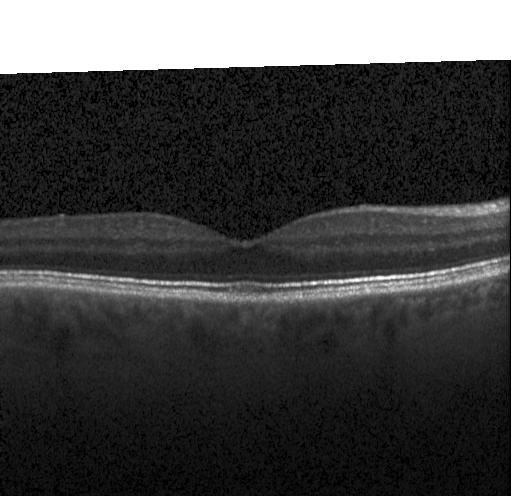

Heidelberg Spectralis OCT system · retinal OCT B-scan. Finding: neither CNV, DME, nor drusen.